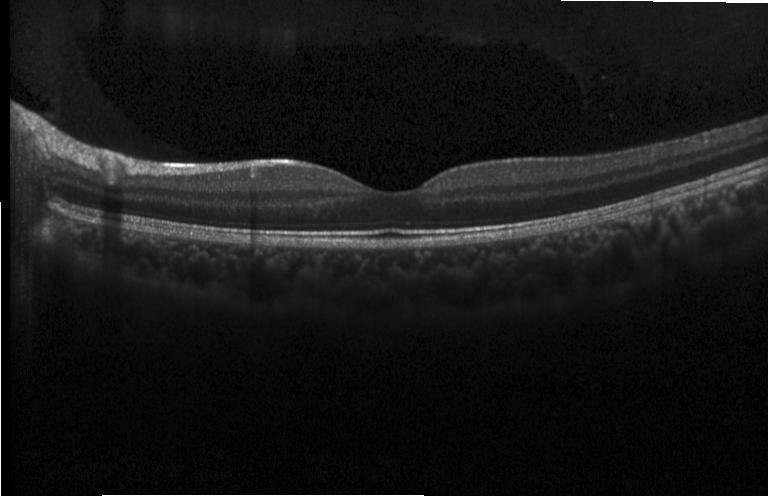
Diagnosis: neither choroidal neovascularization, diabetic macular edema, nor drusen.